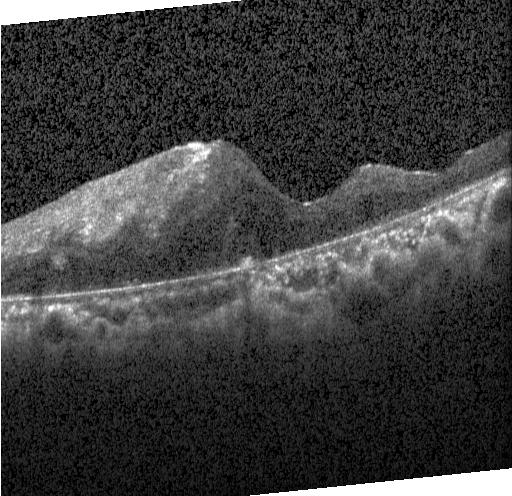
Instrument: Heidelberg Spectralis · through the macula · OCT B-scan · SD-OCT. OCT finding: choroidal neovascularization.